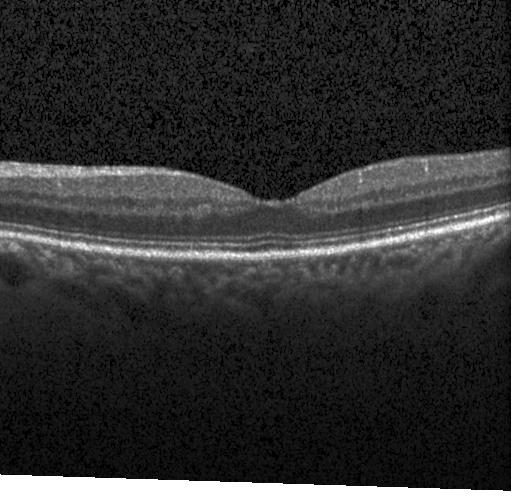
SD-OCT. Retinal OCT cross-section.
Diagnosis: no evidence of choroidal neovascularization, diabetic macular edema, or drusen.